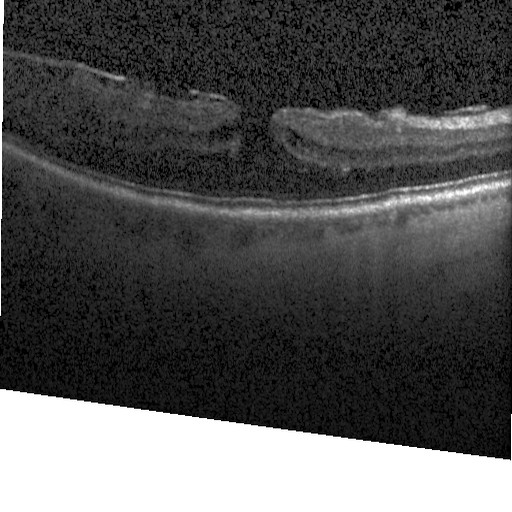
Spectral-domain optical coherence tomography · optical coherence tomography B-scan · instrument: Heidelberg Spectralis.
DME.